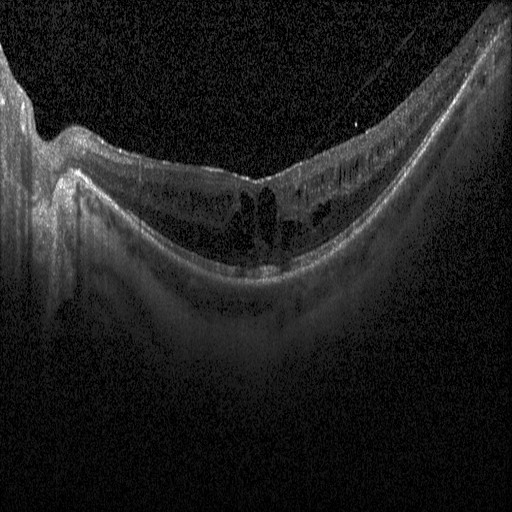

Optical coherence tomography B-scan · SD-OCT · fovea-centered
Diagnosis: diabetic macular edema (DME).